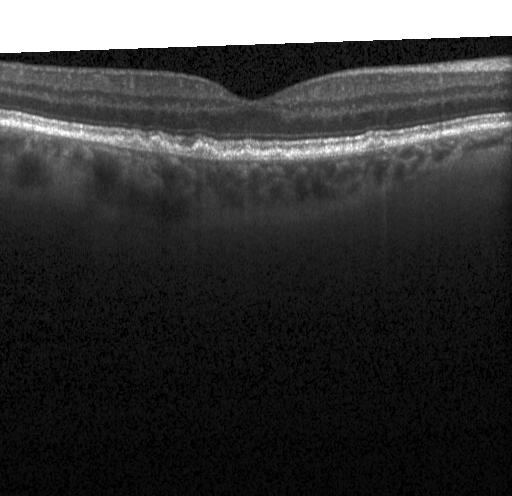
Dx: drusen.